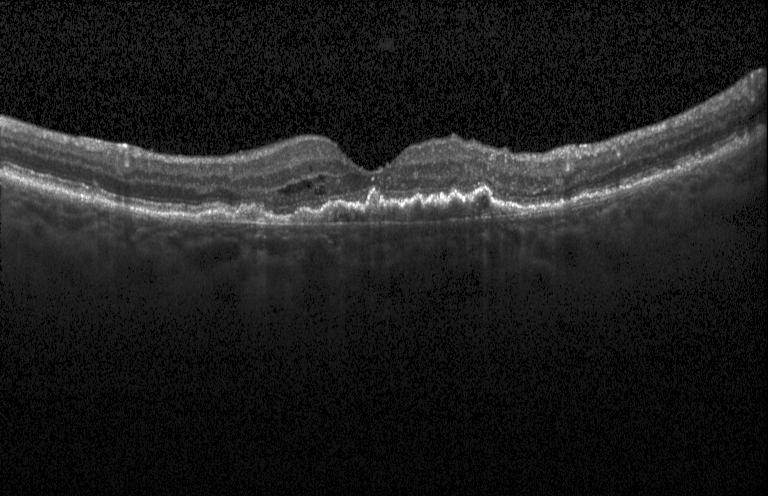 Spectral-domain OCT · optical coherence tomography B-scan
Assessment: a choroidal neovascular membrane.